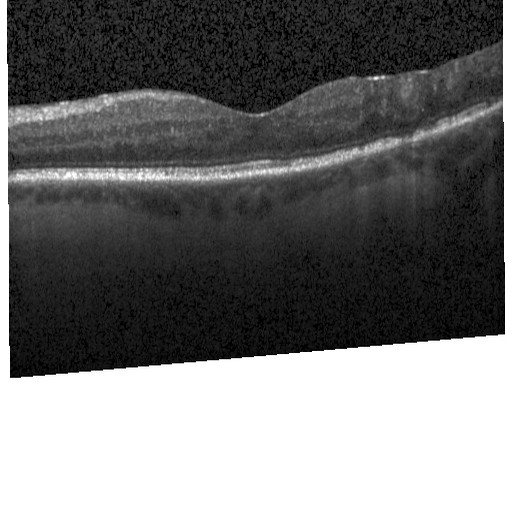

Diagnosis: diabetic macular edema.